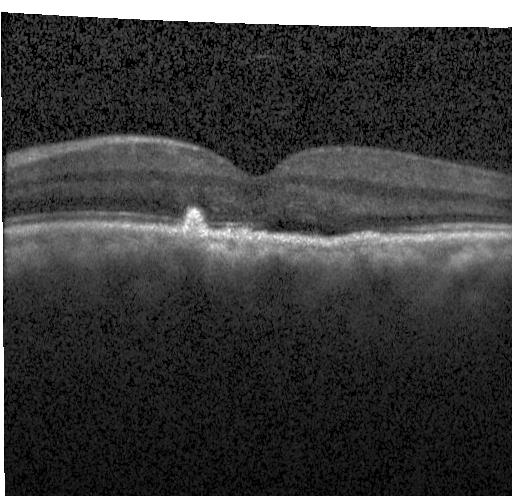
Heidelberg Spectralis, optical coherence tomography scan, SD-OCT, macular scan. Impression: a choroidal neovascular membrane.